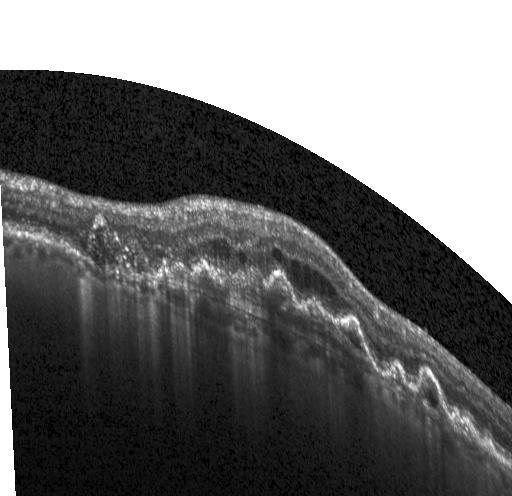

Heidelberg Spectralis. Horizontal scan through the fovea. Optical coherence tomography scan.
Finding: choroidal neovascularization (CNV).